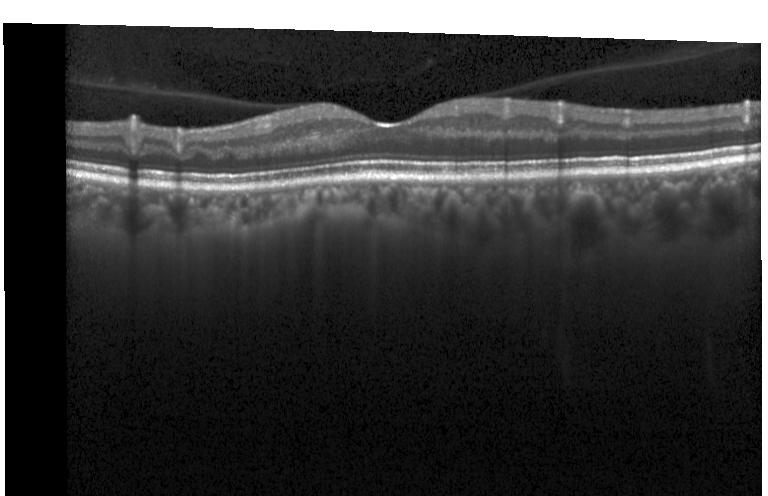 Acquired on a Heidelberg Spectralis. Macular scan. Retinal OCT cross-section.
Diagnosis: no choroidal neovascularization, diabetic macular edema, or drusen.